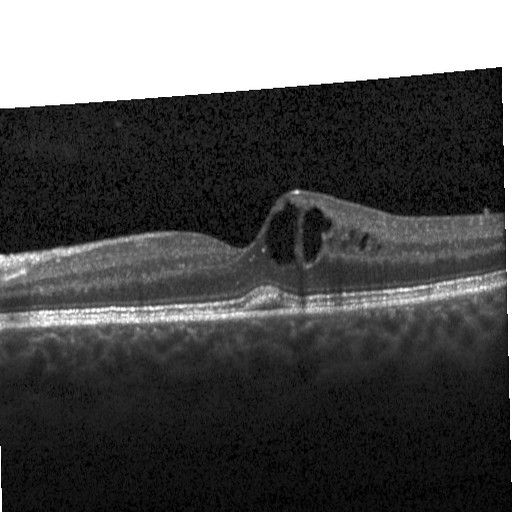

OCT finding: diabetic macular edema (DME).